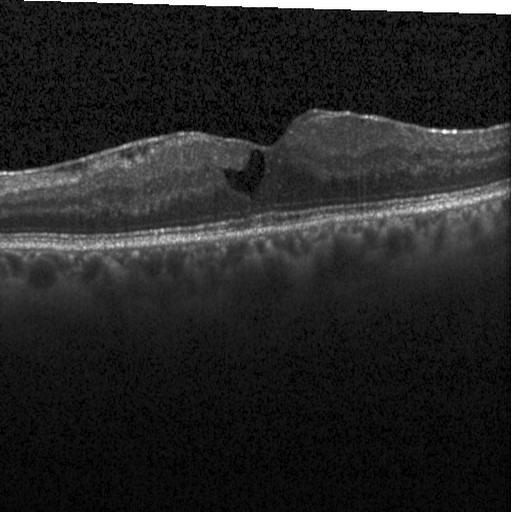 Heidelberg Spectralis OCT system; optical coherence tomography B-scan; SD-OCT; horizontal scan through the fovea
This B-scan demonstrates diabetic macular edema.